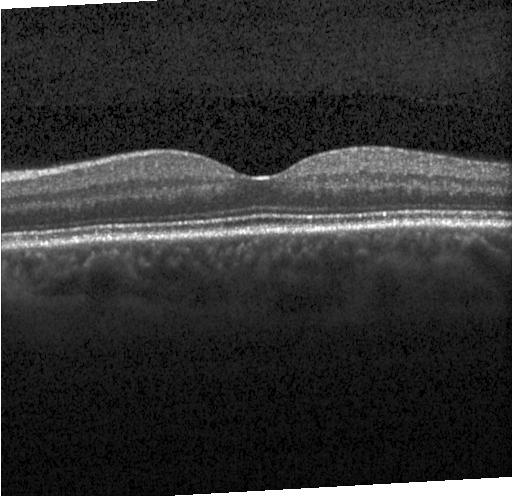
This B-scan demonstrates neither choroidal neovascularization, diabetic macular edema, nor drusen.